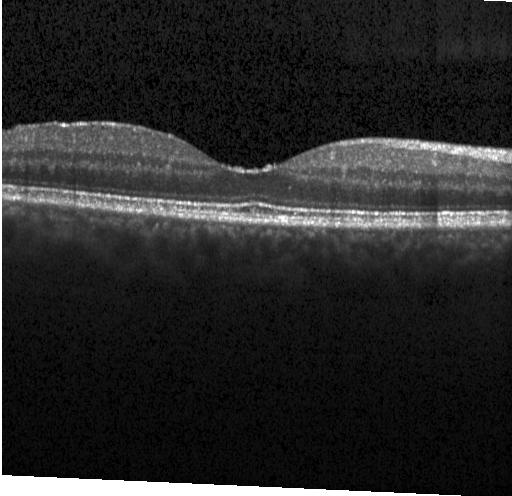
SD-OCT; centered on the fovea; Heidelberg Spectralis; OCT B-scan — Macular OCT: no choroidal neovascularization, diabetic macular edema, or drusen.